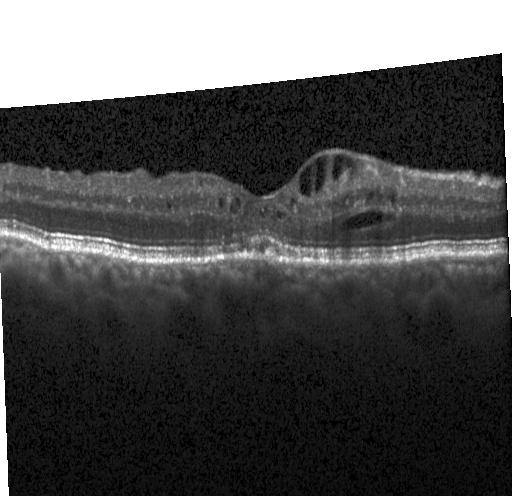
Diagnosis: DME.